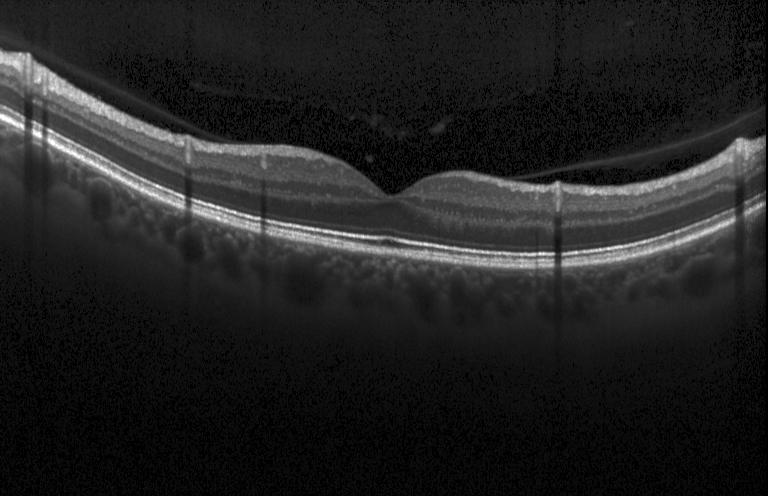
Retinal OCT B-scan — Assessment: no choroidal neovascularization, no diabetic macular edema, and no drusen.